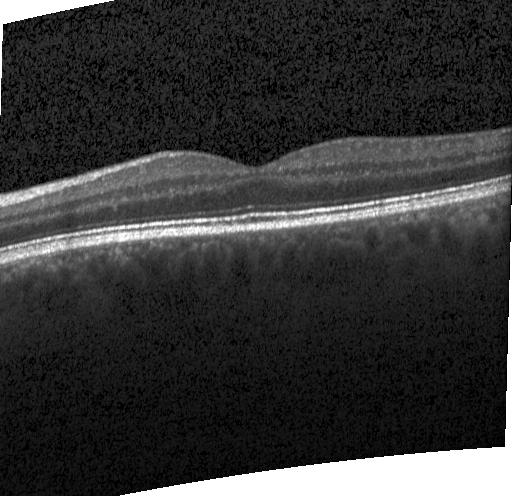

Assessment: neither choroidal neovascularization, diabetic macular edema, nor drusen.